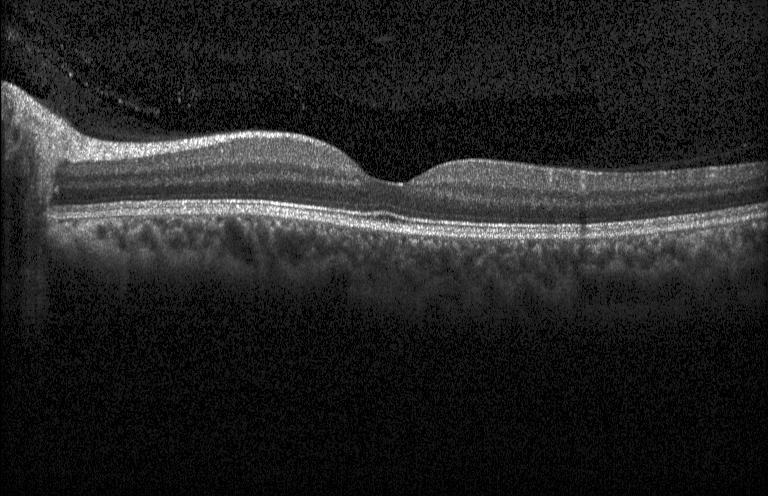

No choroidal neovascularization, no diabetic macular edema, and no drusen.